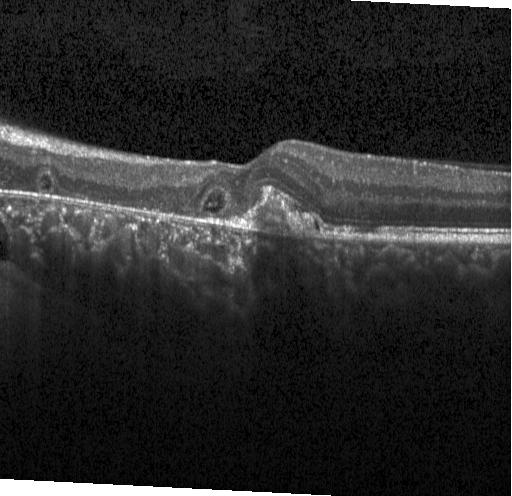

OCT B-scan — Impression: choroidal neovascularization.